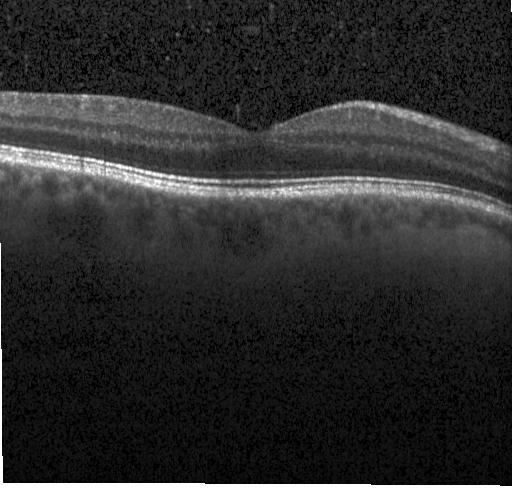

Finding: no evidence of CNV, DME, or drusen.